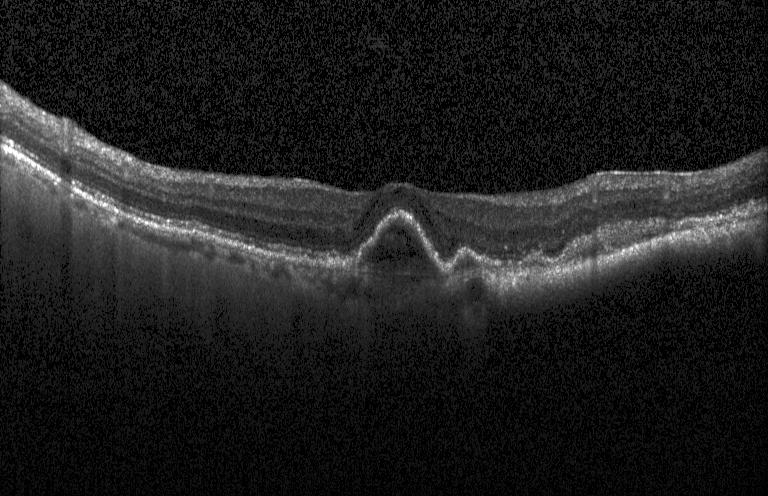
Optical coherence tomography scan; Heidelberg Spectralis; SD-OCT — The scan shows CNV.